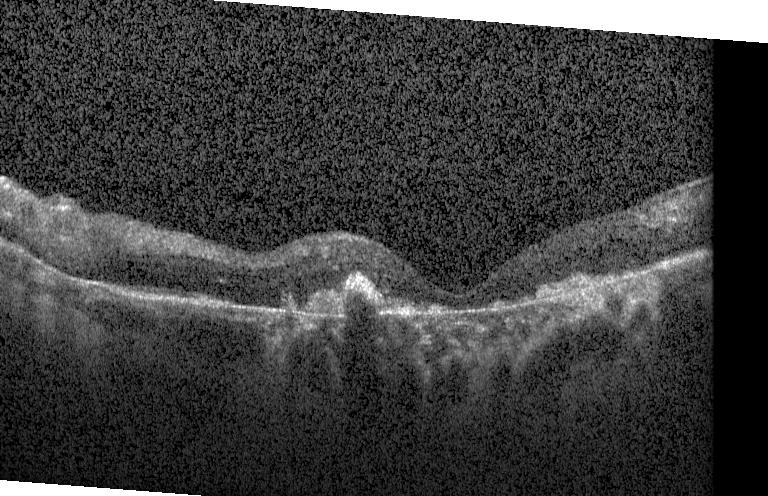

Finding: choroidal neovascularization (CNV).